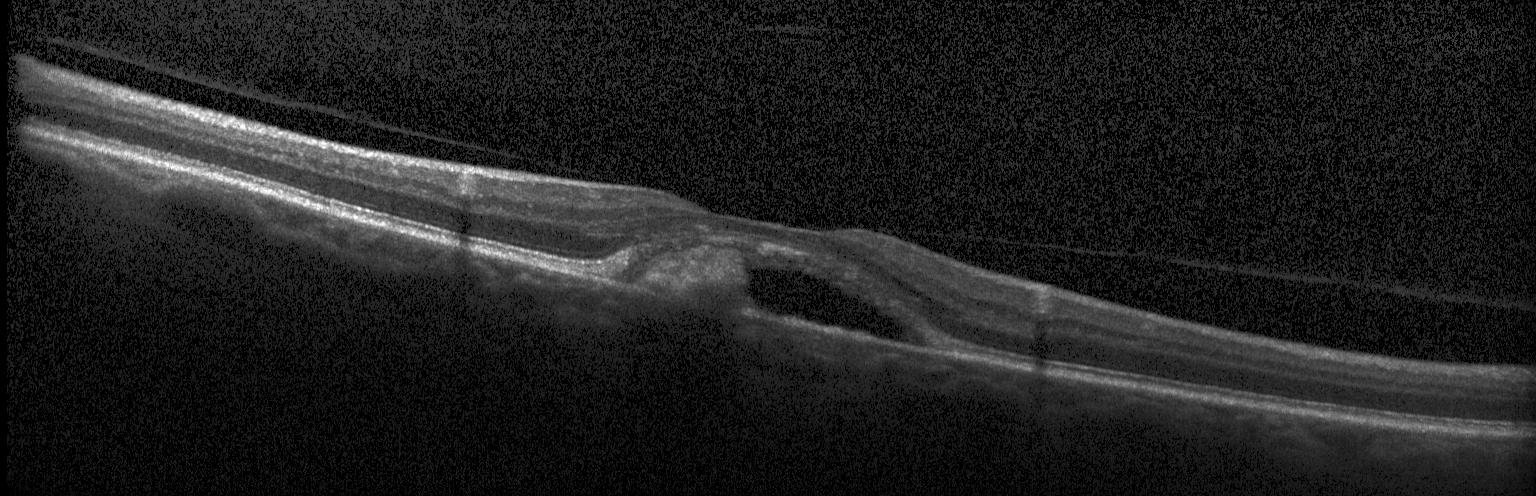 OCT B-scan showing a choroidal neovascular membrane.